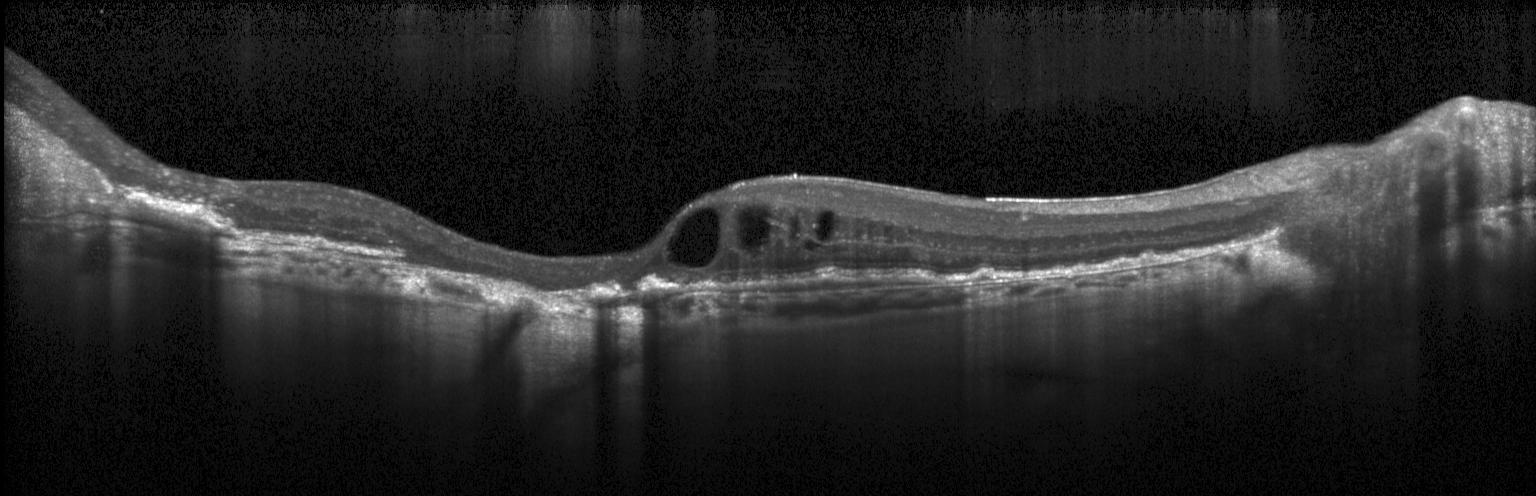 Impression: a choroidal neovascular membrane.